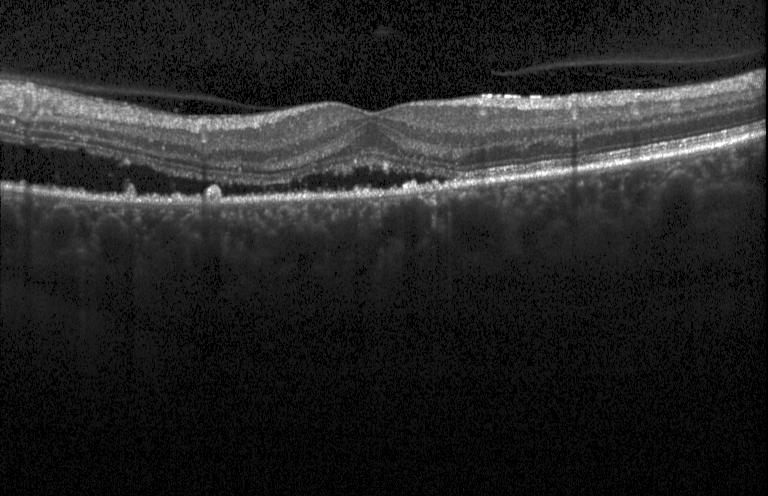

Dx: a choroidal neovascular membrane.